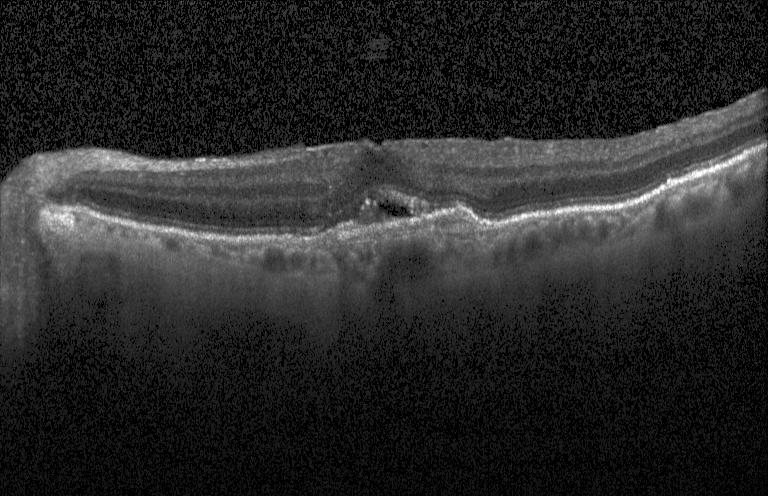 Assessment: choroidal neovascularization (CNV).